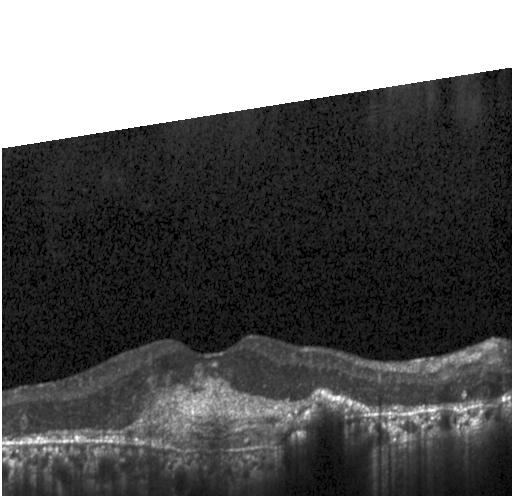

OCT finding: a choroidal neovascular membrane.